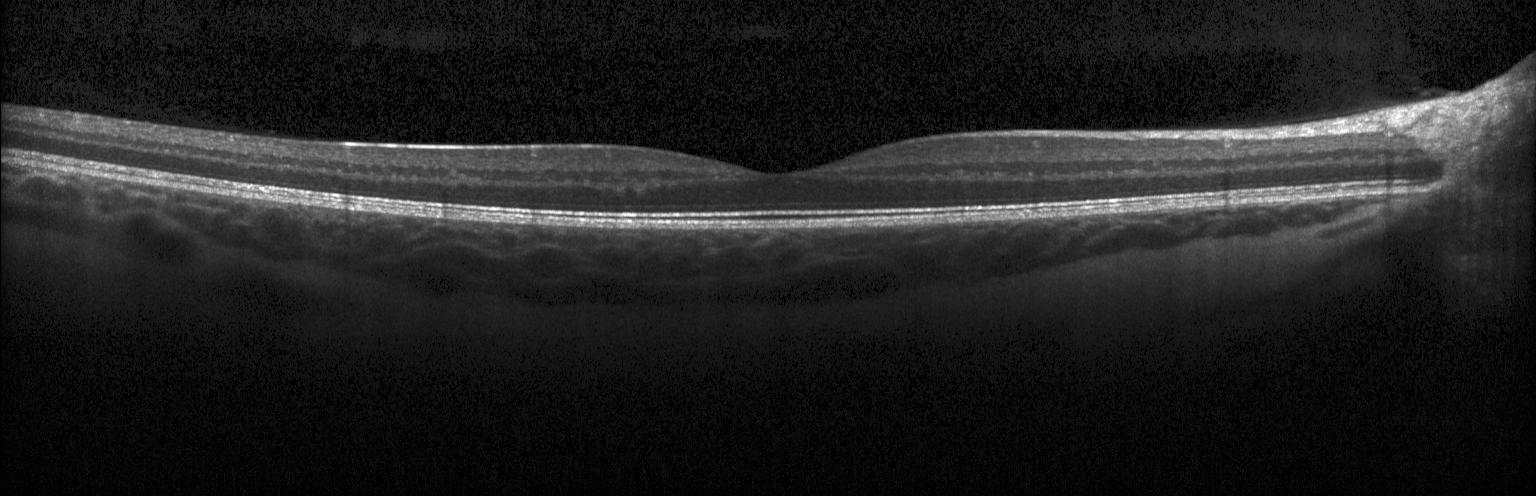

Horizontal scan through the fovea, OCT line scan. The scan shows no choroidal neovascularization, diabetic macular edema, or drusen.